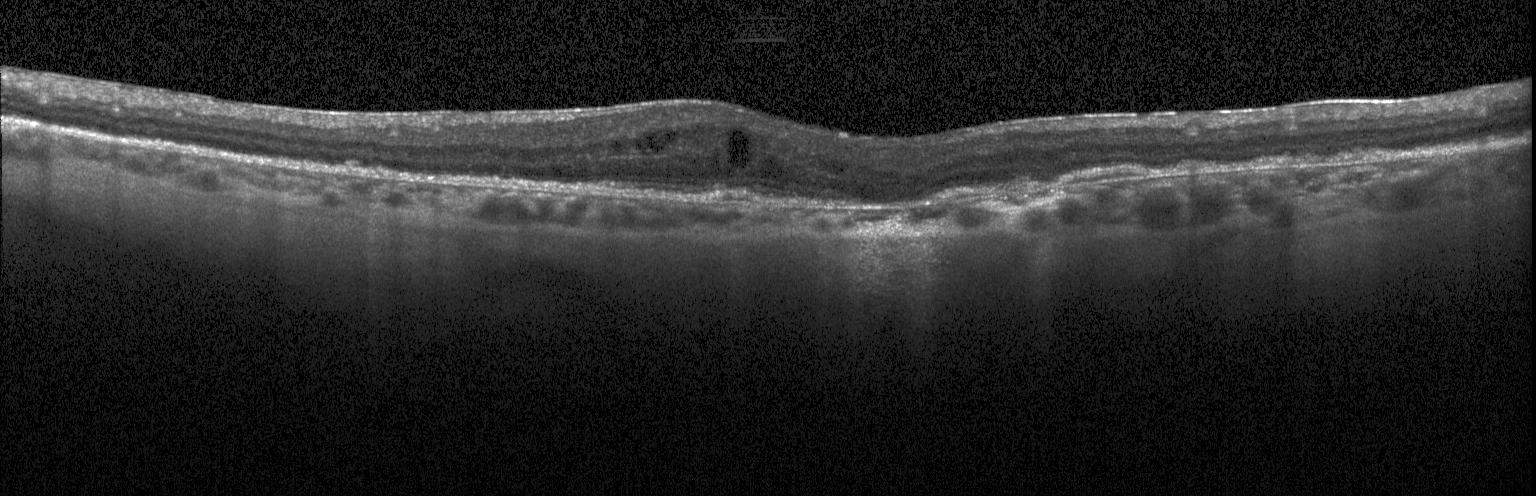

A choroidal neovascular membrane.